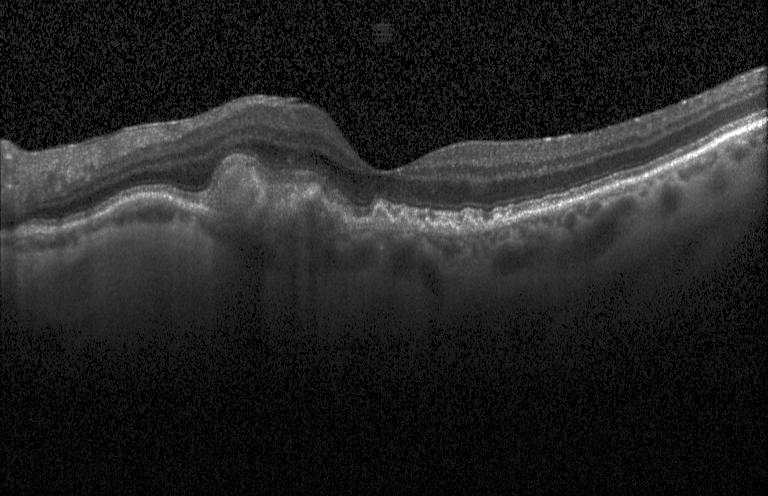
Optical coherence tomography scan.
Dx: choroidal neovascularization (CNV).